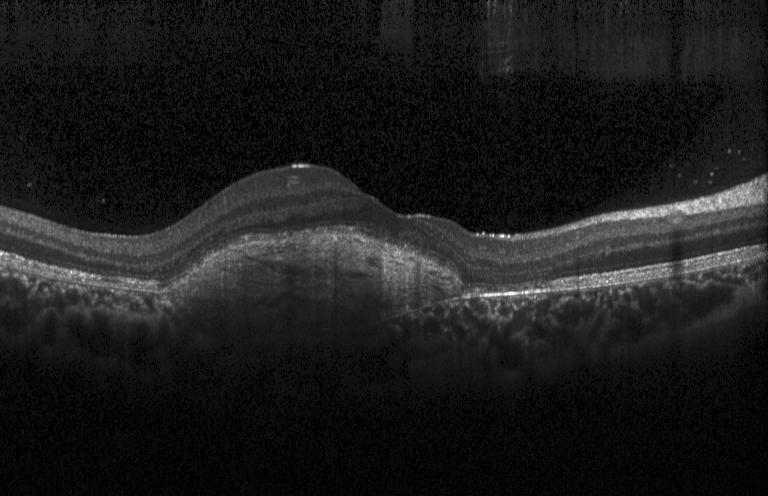 Retinal OCT cross-section
This B-scan demonstrates CNV.